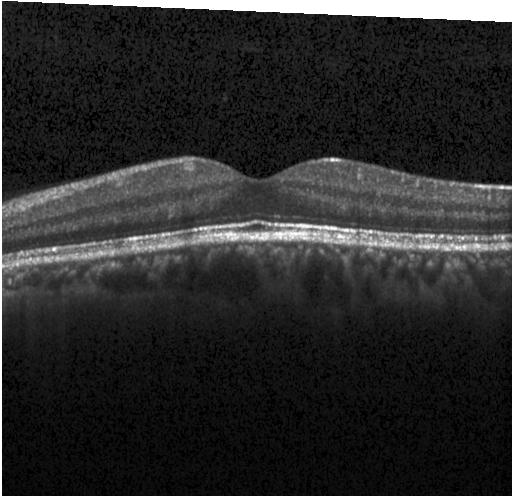 Optical coherence tomography scan, Heidelberg Spectralis, fovea-centered — The scan shows neither CNV, DME, nor drusen.